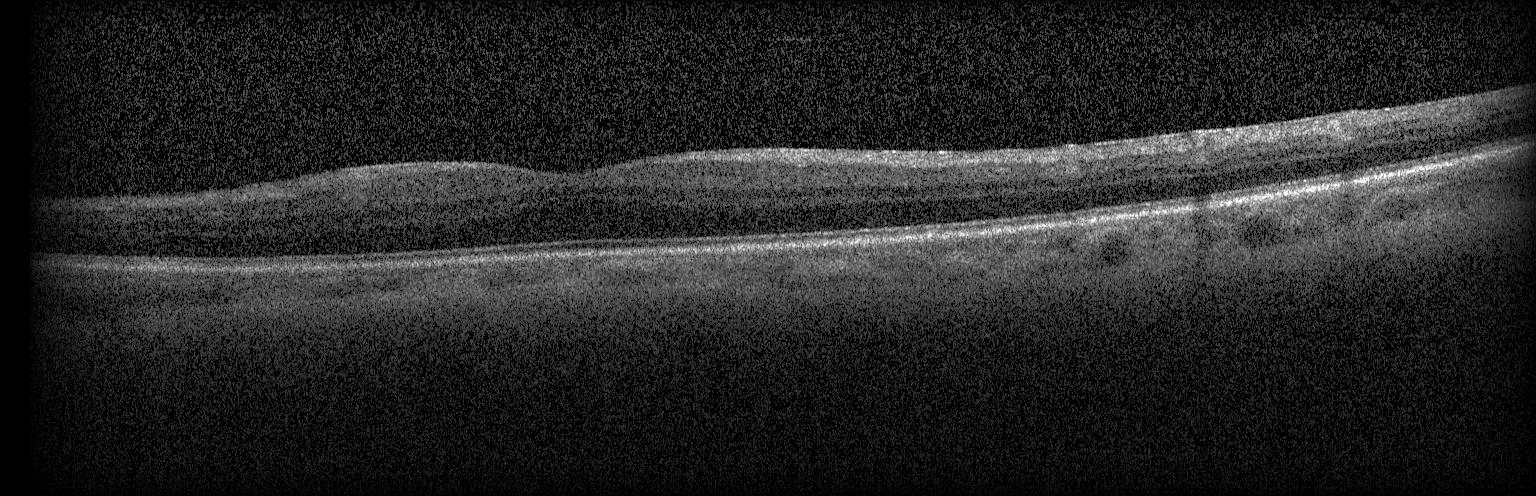
Impression: no choroidal neovascularization, diabetic macular edema, or drusen.